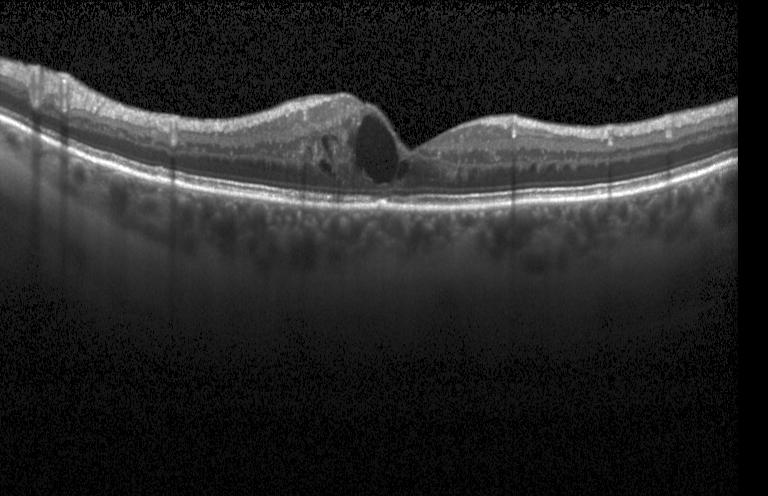

Optical coherence tomography B-scan. Dx: diabetic macular edema.